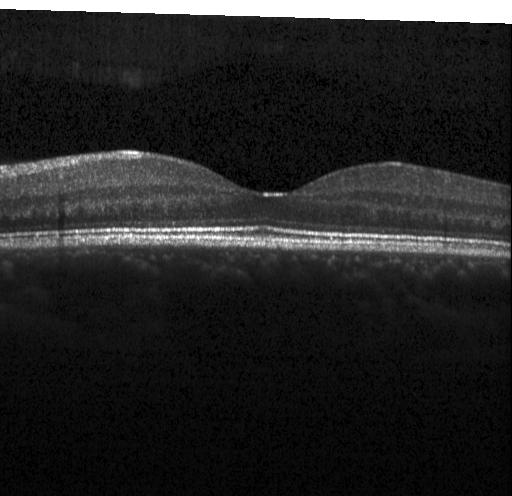
Spectral-domain OCT. Retinal OCT cross-section. Fovea-centered.
This B-scan demonstrates no choroidal neovascularization, no diabetic macular edema, and no drusen.